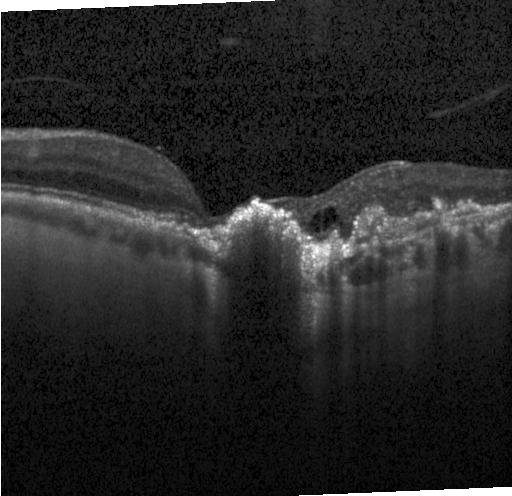
Diagnosis: choroidal neovascularization.